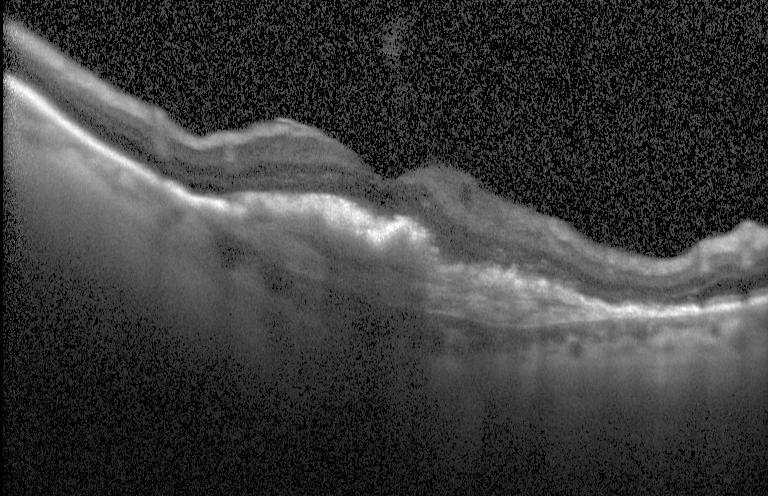
The scan shows a choroidal neovascular membrane.